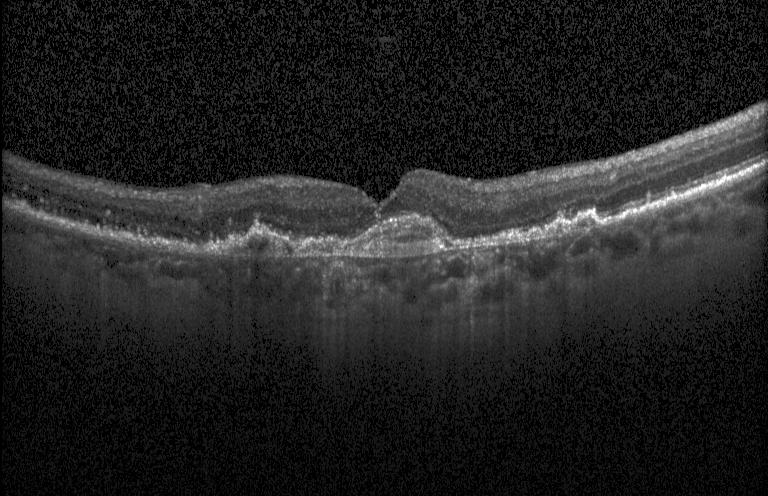
Retinal OCT cross-section
Impression: CNV.